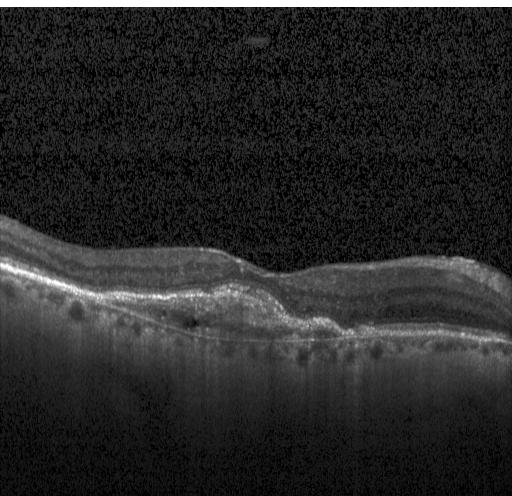

SD-OCT. Retinal OCT B-scan.
This B-scan demonstrates a choroidal neovascular membrane.